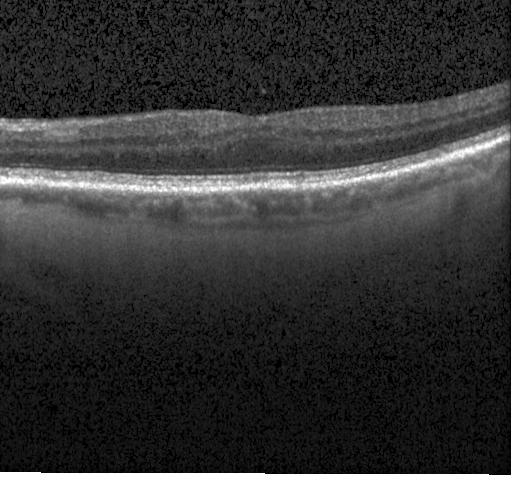
Fovea-centered, instrument: Heidelberg Spectralis, spectral-domain OCT, optical coherence tomography B-scan.
Finding: neither choroidal neovascularization, diabetic macular edema, nor drusen.